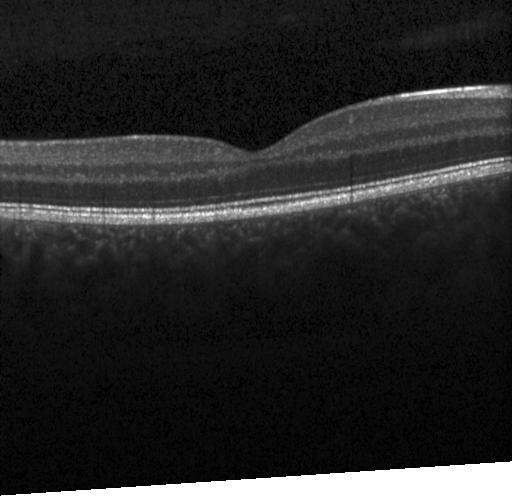 Spectral-domain OCT B-scan: no CNV, DME, or drusen.